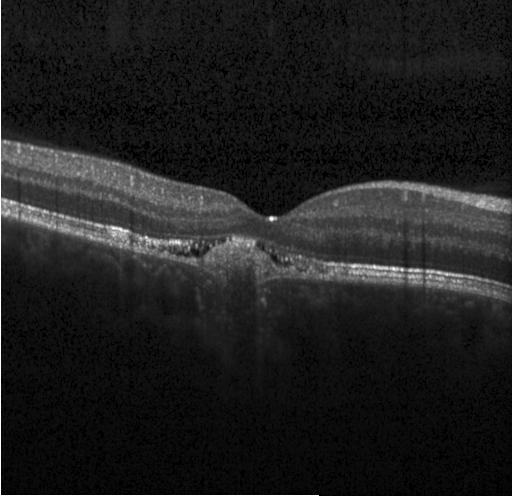

OCT B-scan; spectral-domain OCT. This B-scan demonstrates choroidal neovascularization (CNV).